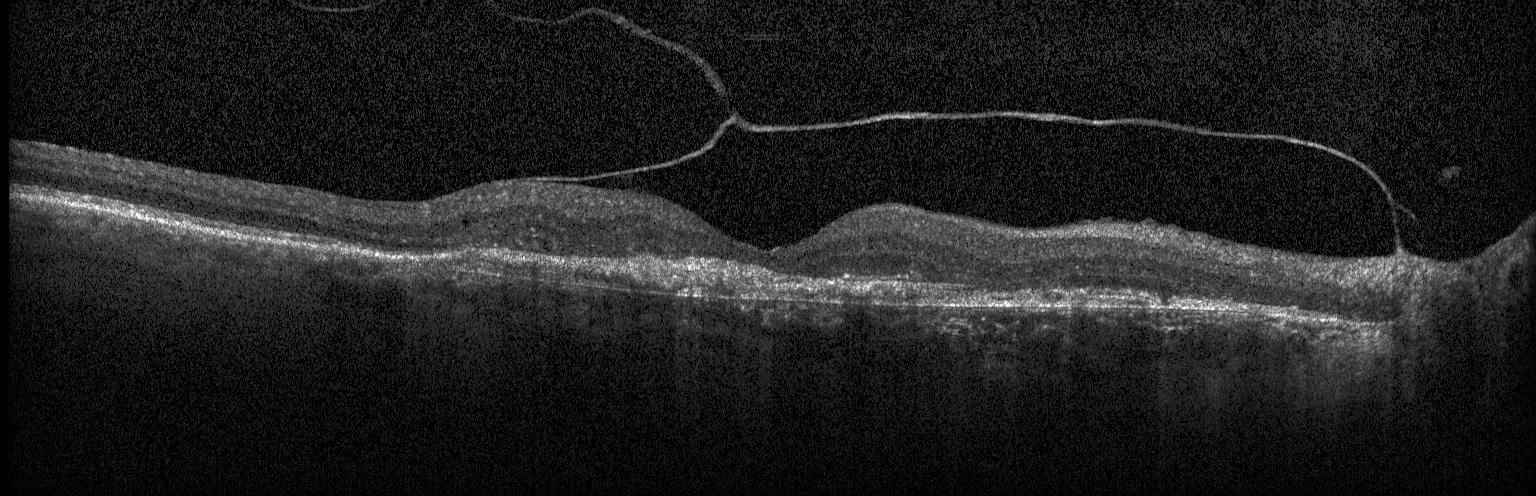 OCT finding: a choroidal neovascular membrane.